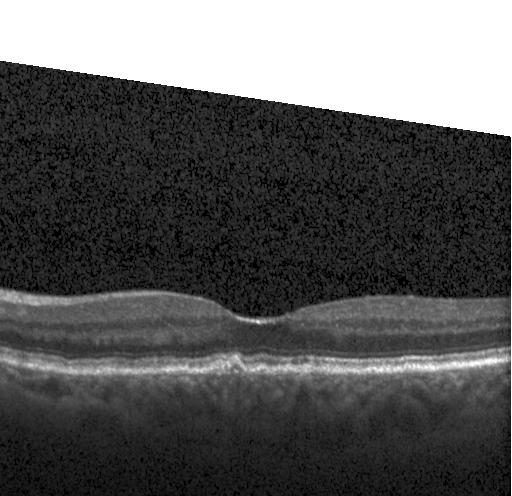

Finding: drusen.